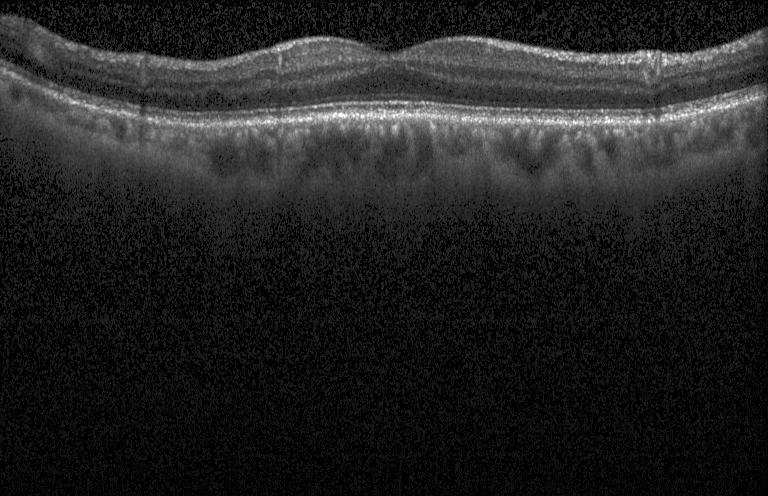 OCT B-scan showing neither choroidal neovascularization, diabetic macular edema, nor drusen.